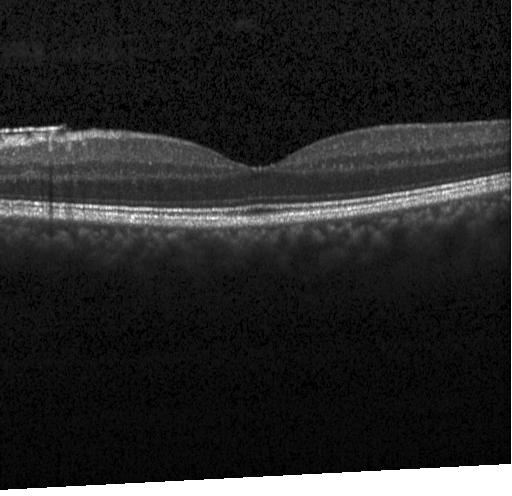
OCT B-scan; macular scan; SD-OCT — Diagnosis: neither choroidal neovascularization, diabetic macular edema, nor drusen.